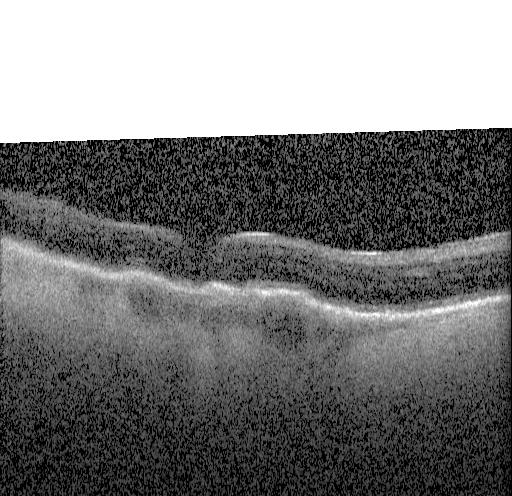 Optical coherence tomography B-scan; SD-OCT.
OCT finding: a choroidal neovascular membrane.